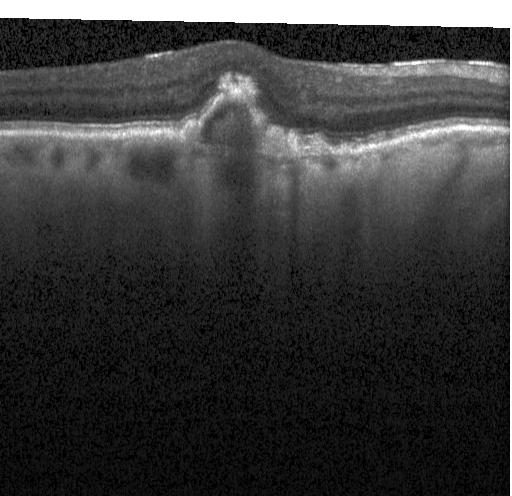

The scan shows choroidal neovascularization.